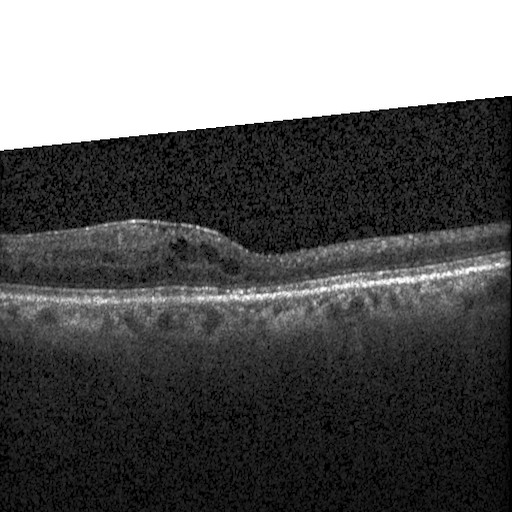

Spectral-domain optical coherence tomography. Retinal OCT B-scan. Heidelberg Spectralis OCT system. OCT finding: DME.